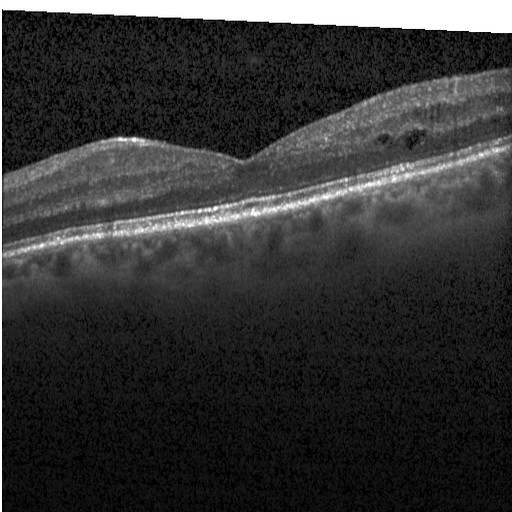 Fovea-centered; acquired on a Heidelberg Spectralis; optical coherence tomography scan — Finding: diabetic macular edema.